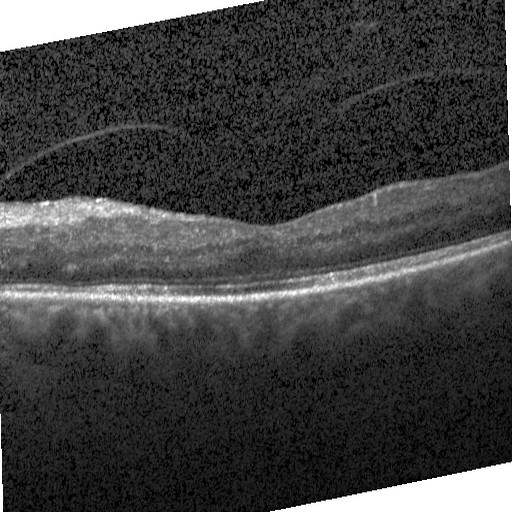 Retinal OCT cross-section, instrument: Heidelberg Spectralis, centered on the fovea.
Dx: DME.